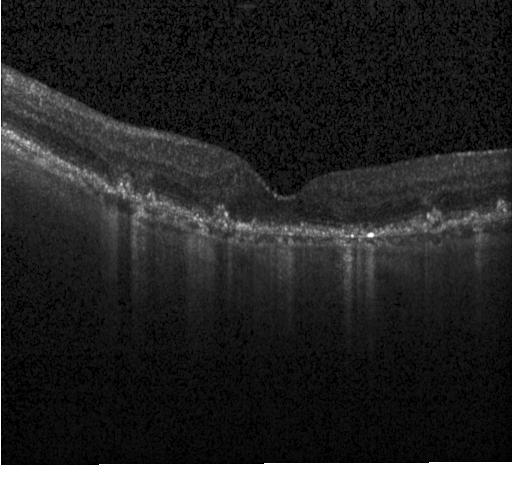

Spectral-domain OCT · optical coherence tomography B-scan.
OCT finding: a choroidal neovascular membrane.